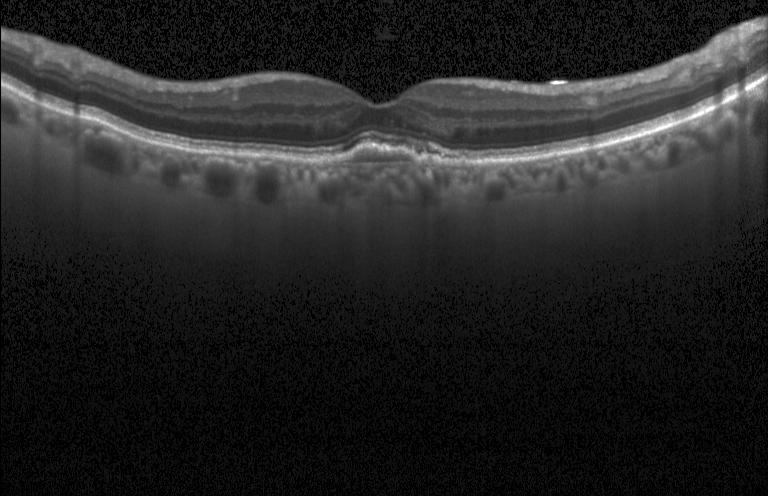

Dx: choroidal neovascularization (CNV).